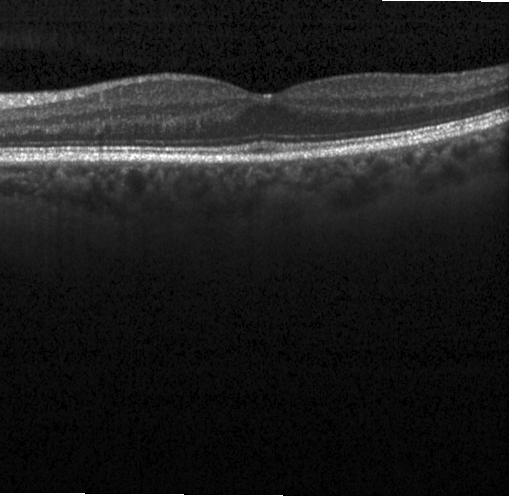 OCT B-scan; horizontal scan through the fovea — This B-scan demonstrates no choroidal neovascularization, diabetic macular edema, or drusen.